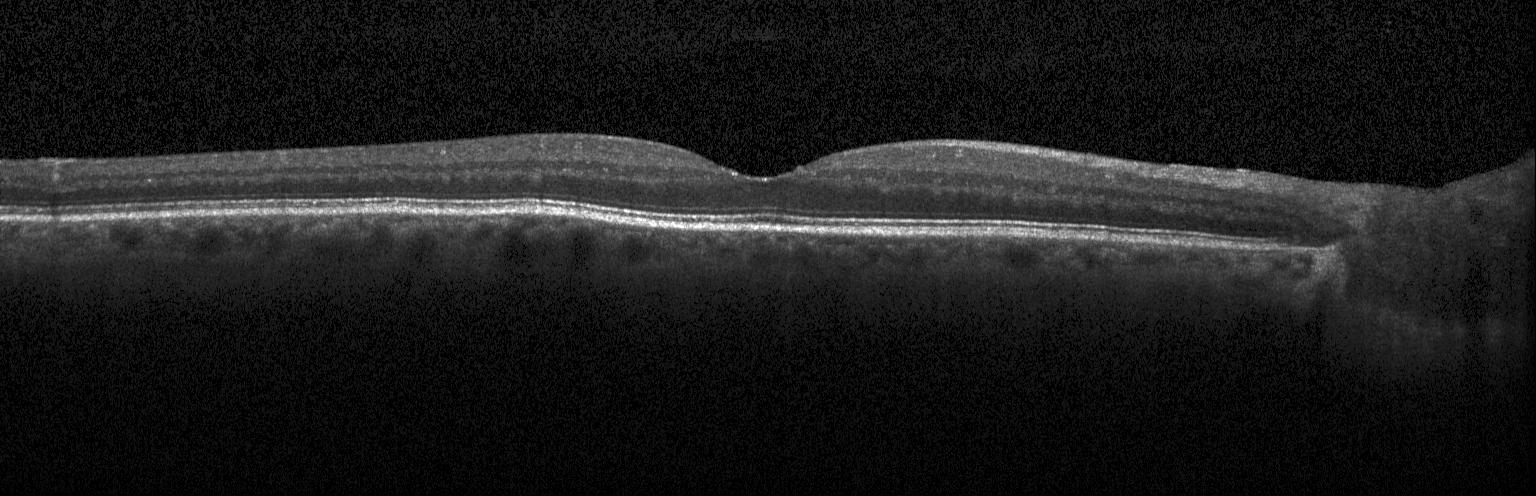 Centered on the fovea. Spectral-domain OCT. OCT line scan. Diagnosis: no evidence of CNV, DME, or drusen.